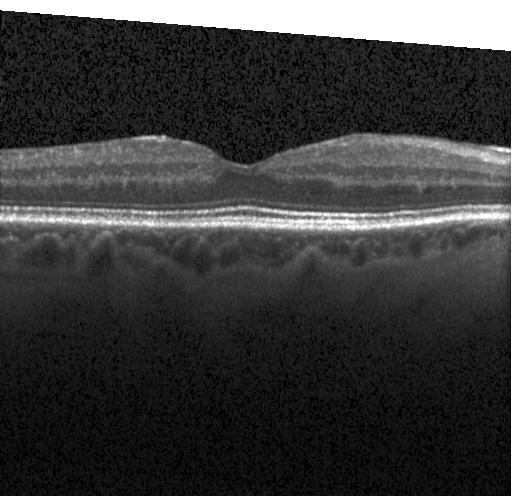 Instrument: Heidelberg Spectralis. OCT B-scan. Macular scan
The scan shows no CNV, DME, or drusen.